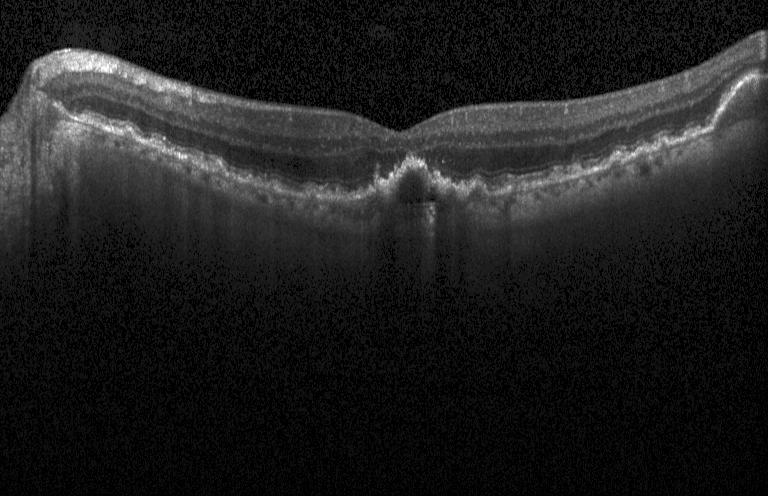

Diagnosis: a choroidal neovascular membrane.